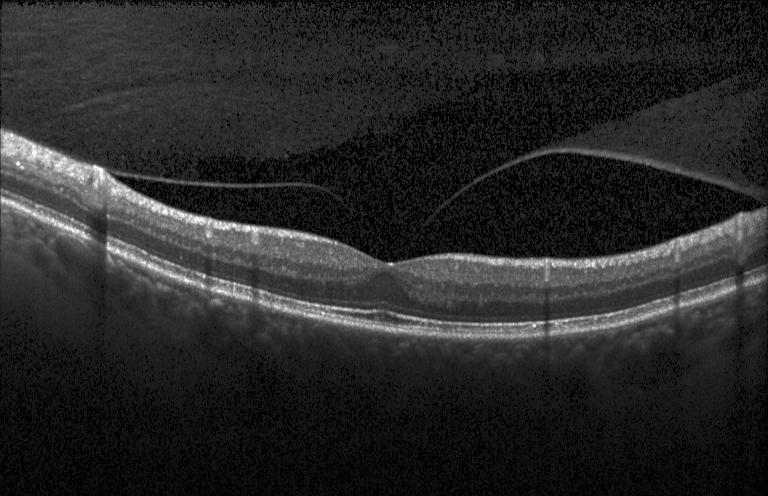 Macular OCT: no CNV, no DME, and no drusen.